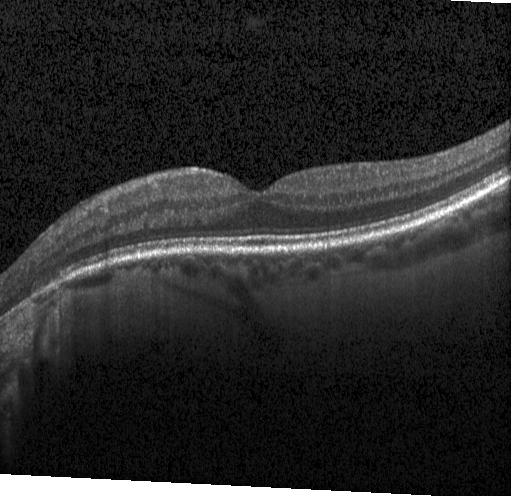
Macular OCT demonstrating no evidence of choroidal neovascularization, diabetic macular edema, or drusen.